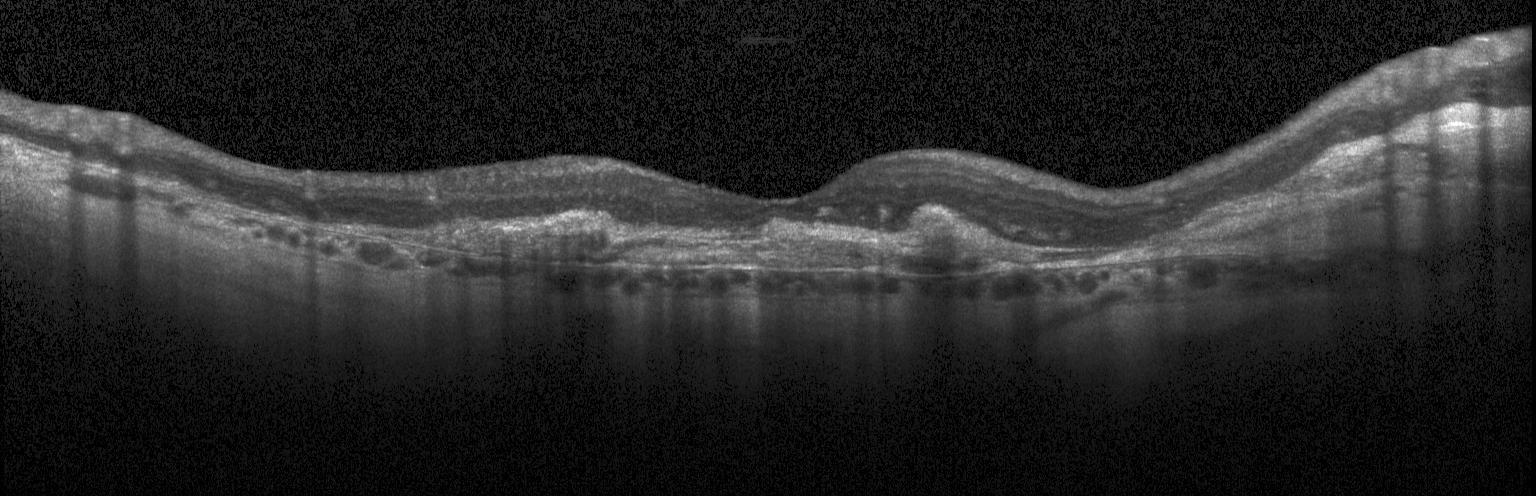

OCT line scan. The scan shows a choroidal neovascular membrane.